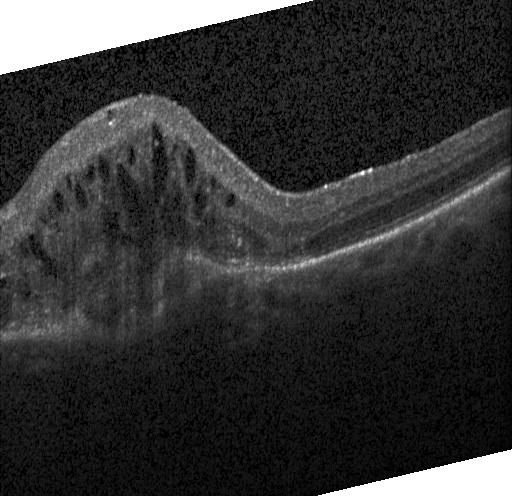
Finding: a choroidal neovascular membrane.